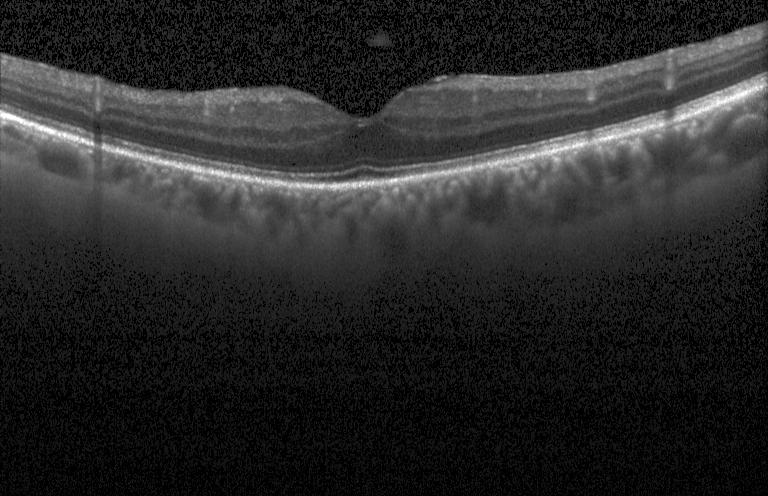
Neither CNV, DME, nor drusen.